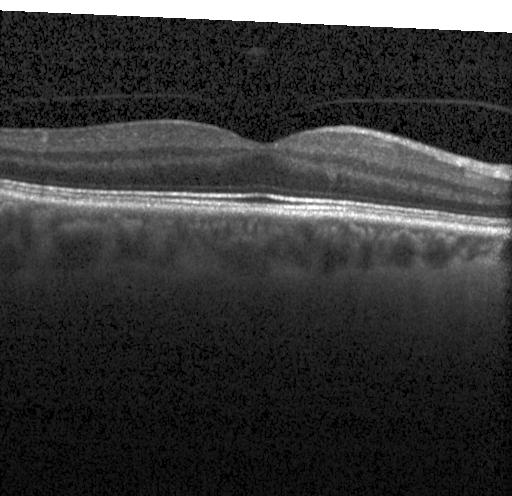
Spectral-domain OCT B-scan: no choroidal neovascularization, no diabetic macular edema, and no drusen.